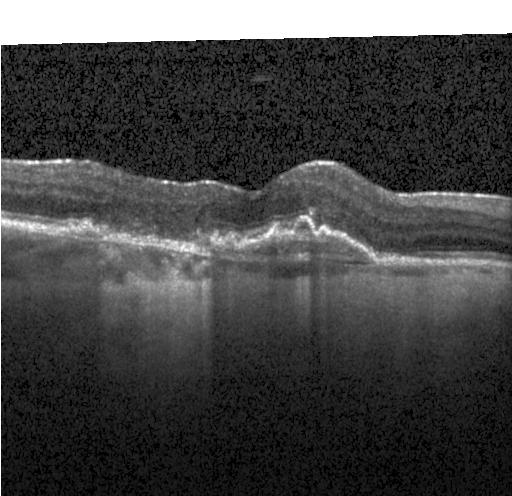
Retinal OCT cross-section.
Finding: a choroidal neovascular membrane.